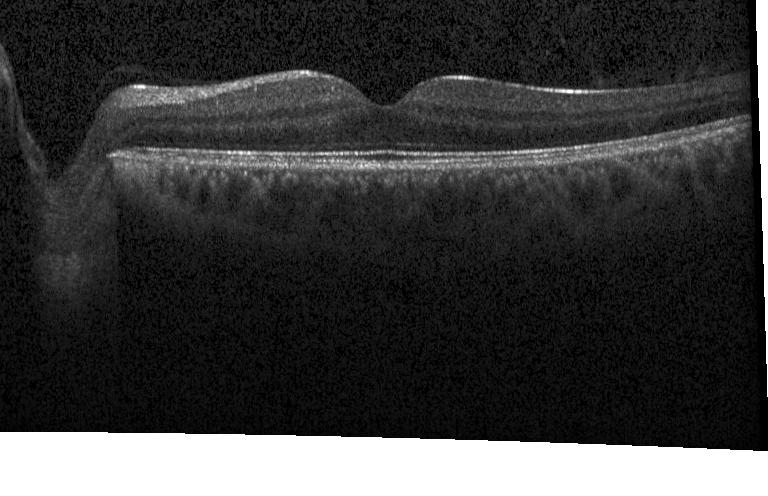 OCT line scan; fovea-centered; spectral-domain optical coherence tomography; Heidelberg Spectralis.
Diagnosis: neither choroidal neovascularization, diabetic macular edema, nor drusen.